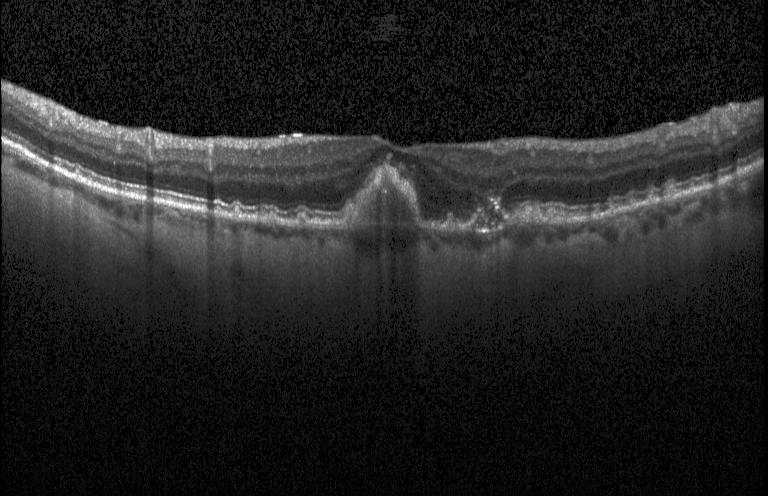
Macular OCT: choroidal neovascularization (CNV).